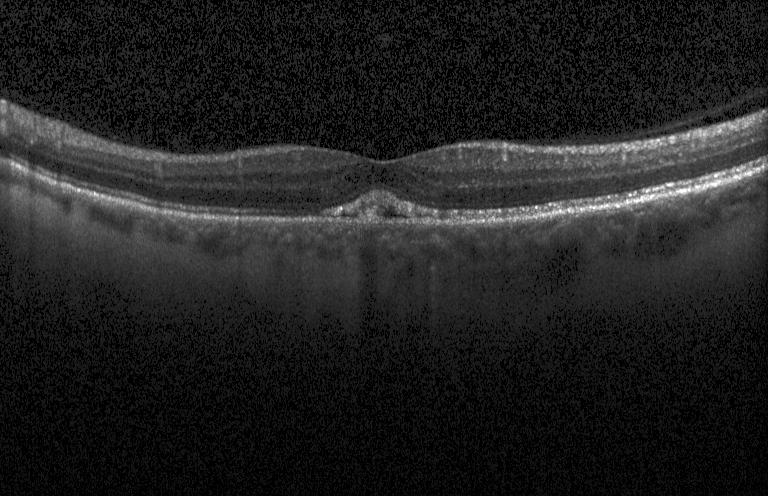
Retinal OCT cross-section — Assessment: choroidal neovascularization.